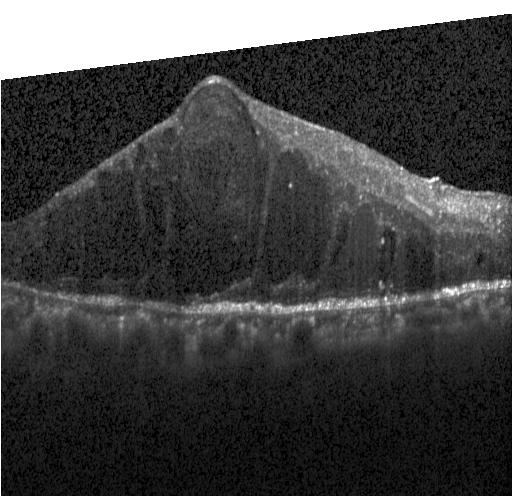

This B-scan demonstrates diabetic macular edema (DME).